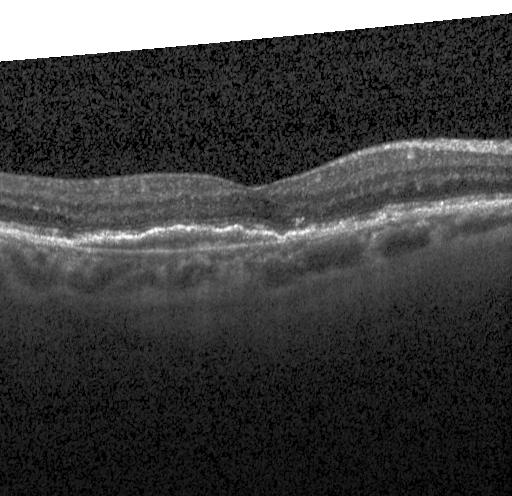
Retinal OCT cross-section showing a choroidal neovascular membrane.